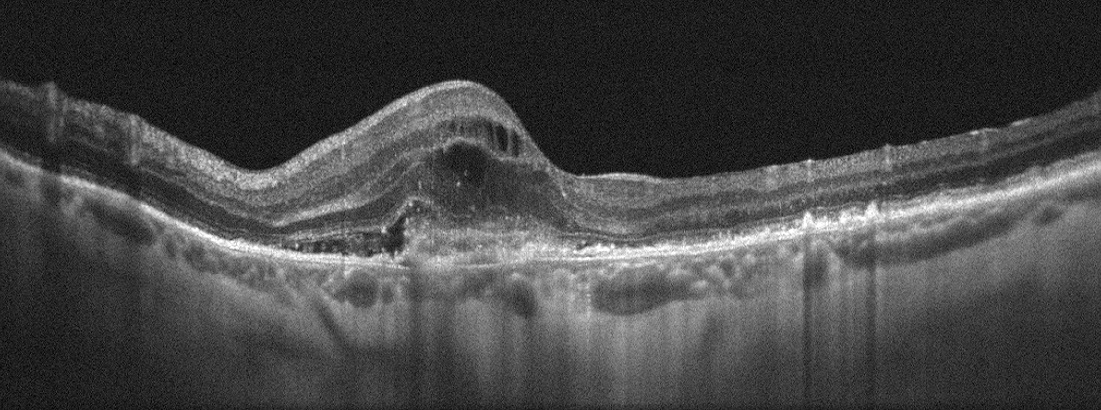
This B-scan demonstrates age-related macular degeneration (AMD).